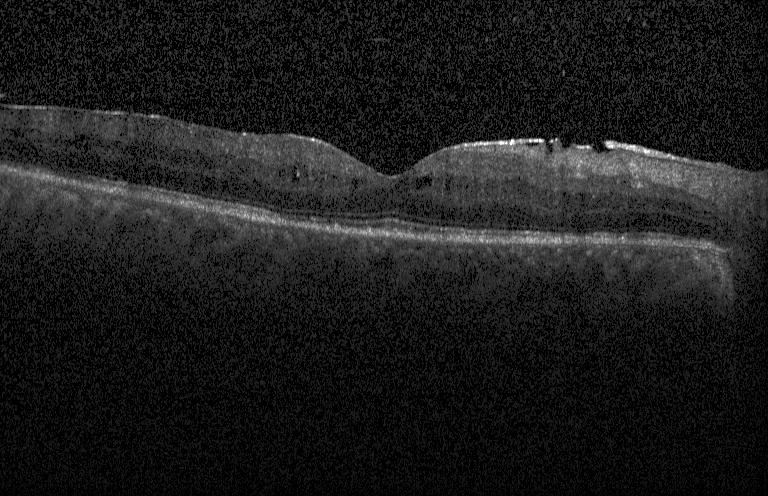
OCT scan showing DME.